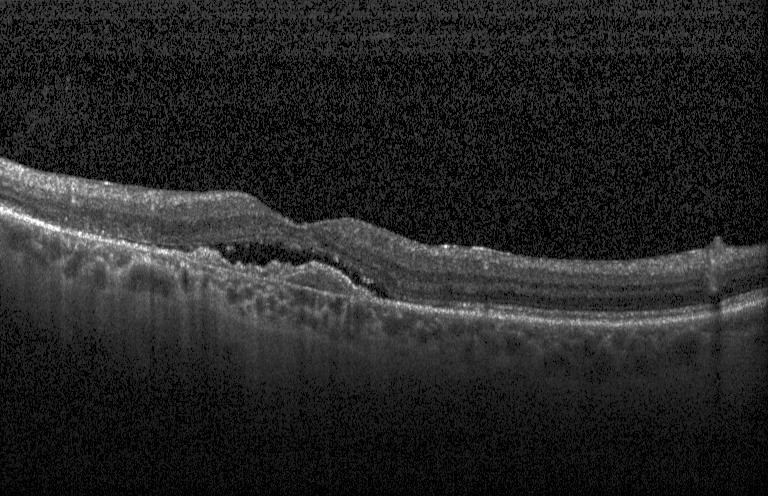
SD-OCT, acquired on a Heidelberg Spectralis, retinal OCT B-scan. Macular OCT: CNV.